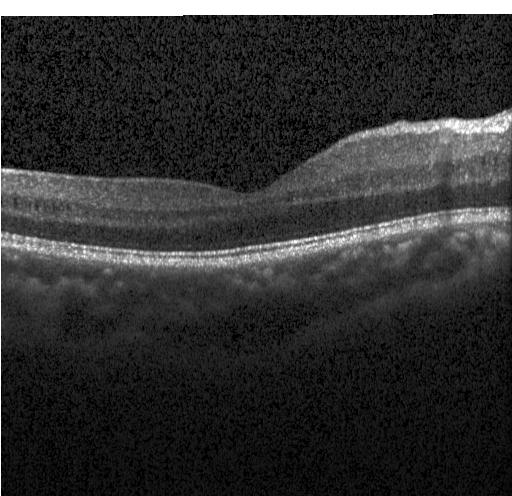
Optical coherence tomography B-scan — This B-scan demonstrates no CNV, DME, or drusen.